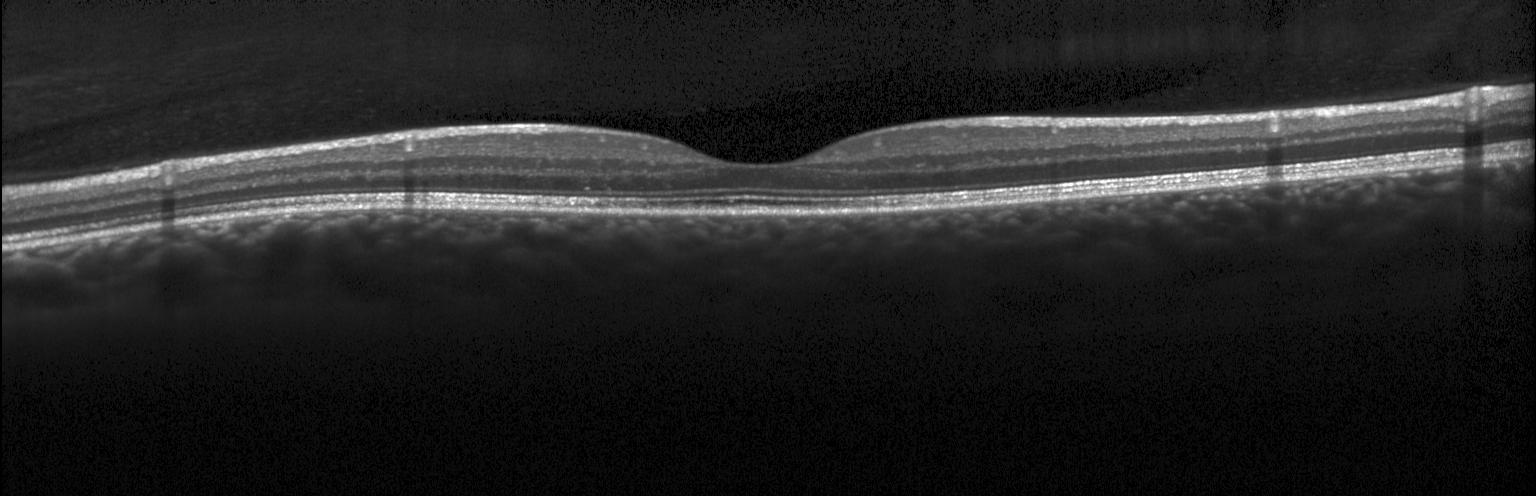 SD-OCT; OCT B-scan
The scan shows neither choroidal neovascularization, diabetic macular edema, nor drusen.